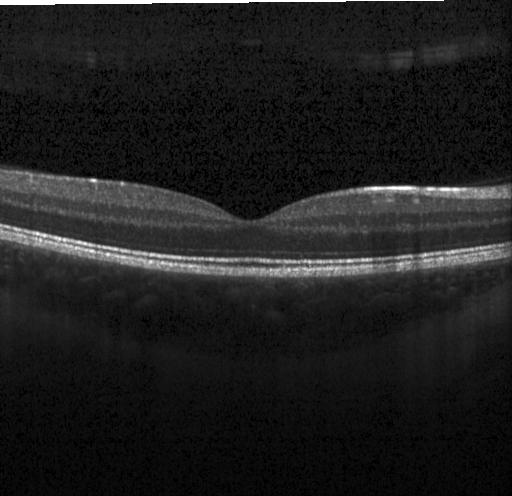
Retinal OCT cross-section showing no choroidal neovascularization, no diabetic macular edema, and no drusen.